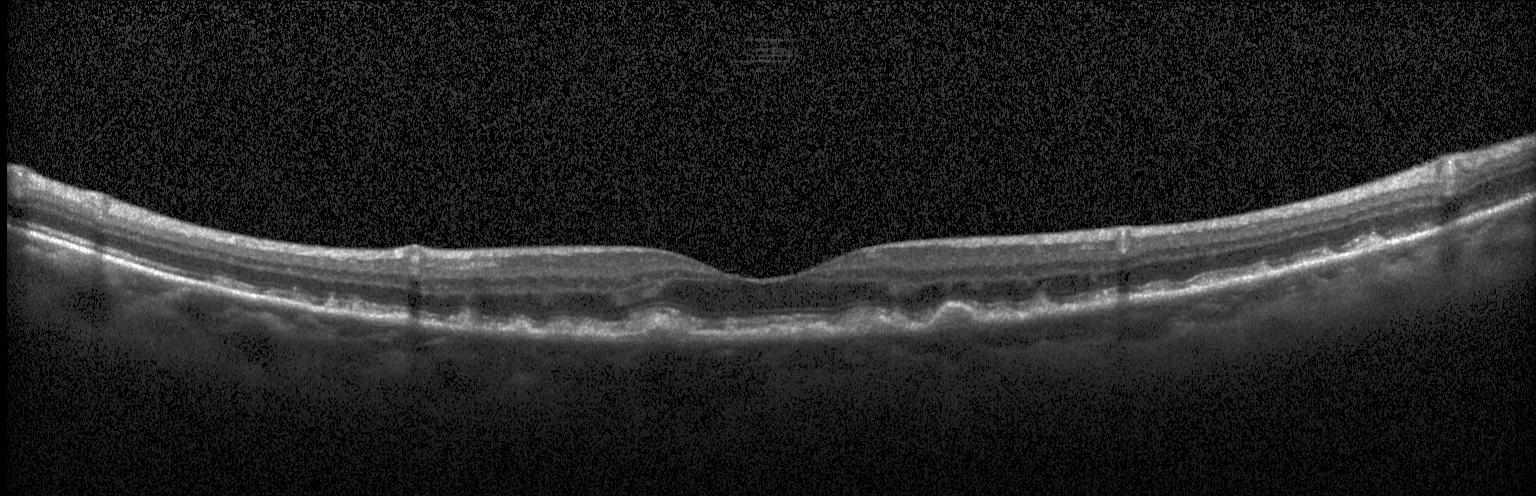
Optical coherence tomography scan, spectral-domain optical coherence tomography. This B-scan demonstrates sub-RPE drusenoid deposits.